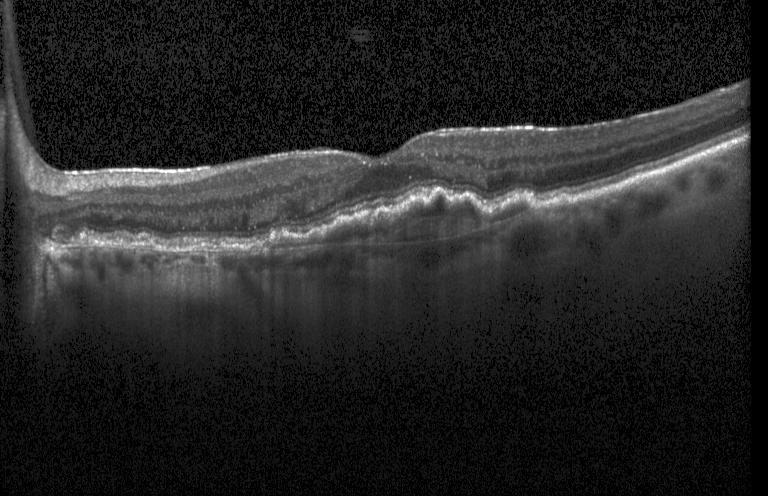

Spectral-domain OCT · OCT B-scan
Diagnosis: CNV.